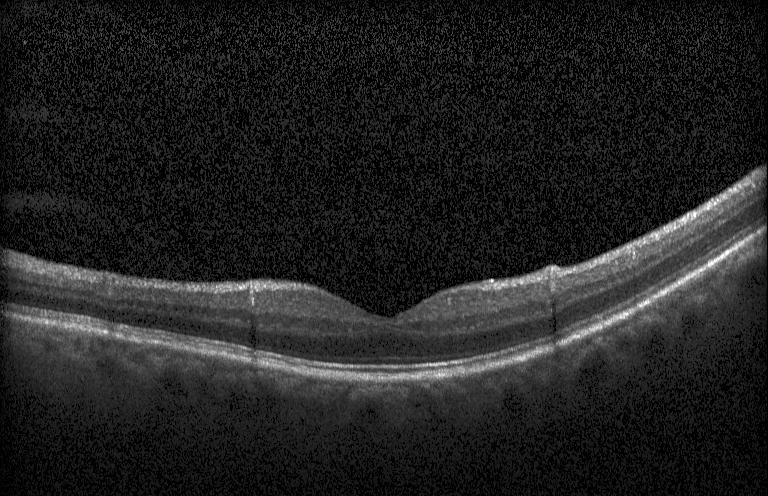
Heidelberg Spectralis OCT system; retinal OCT cross-section — Impression: no choroidal neovascularization, no diabetic macular edema, and no drusen.